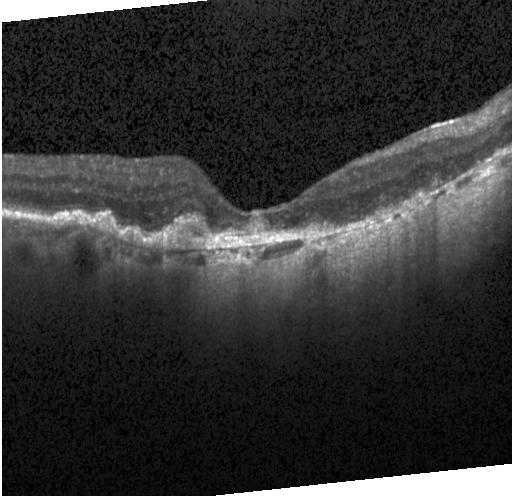
OCT scan showing CNV.